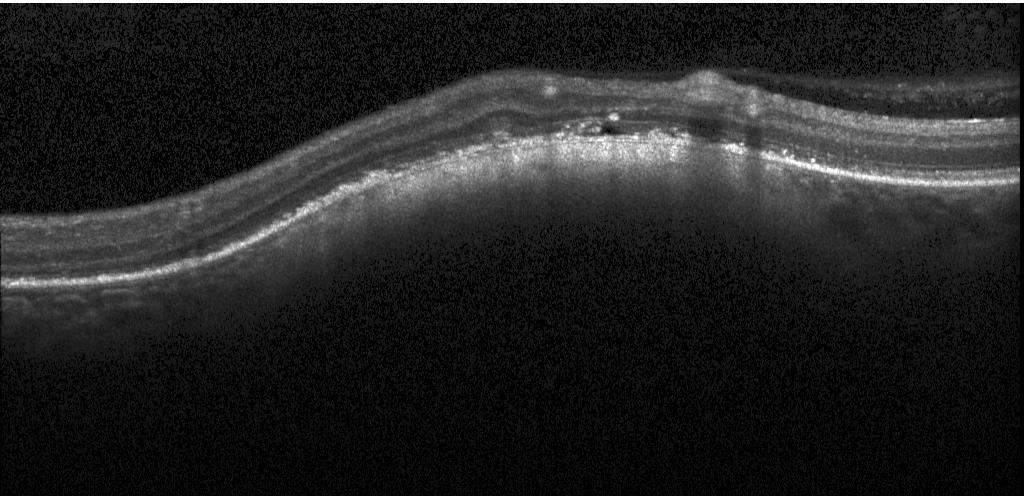
OCT finding: a choroidal neovascular membrane.